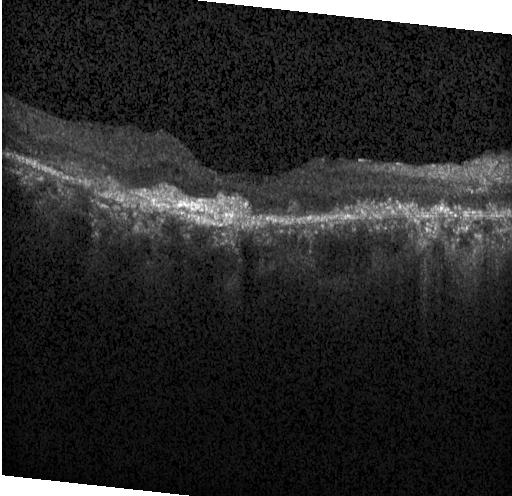 OCT finding: choroidal neovascularization.